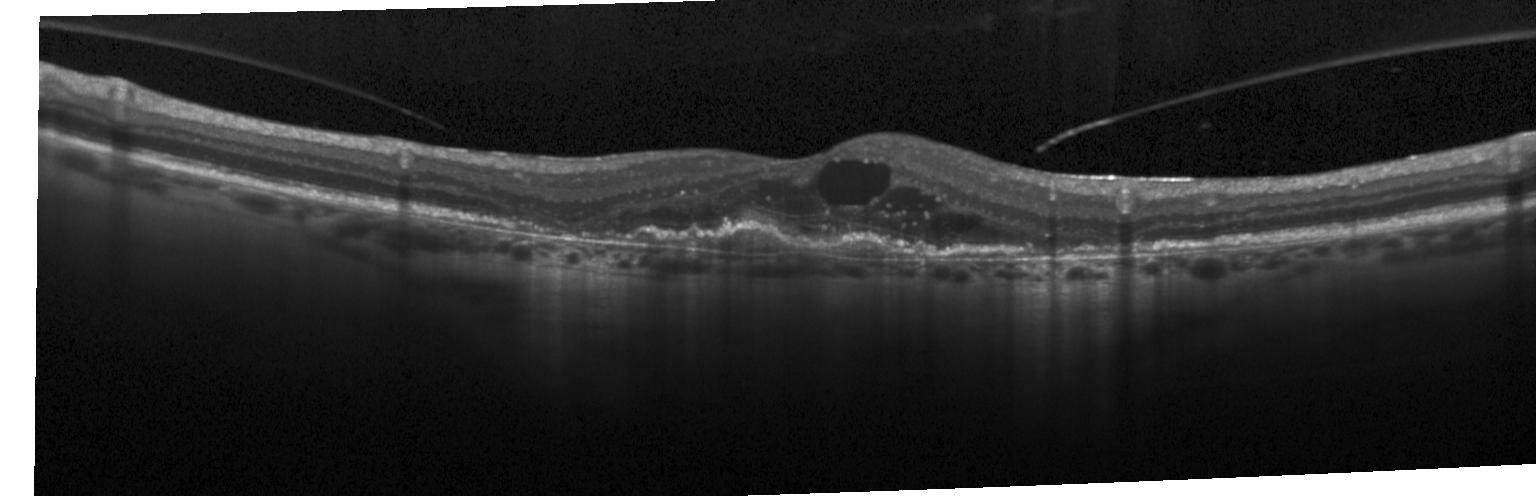

Retinal OCT B-scan. Impression: a choroidal neovascular membrane.